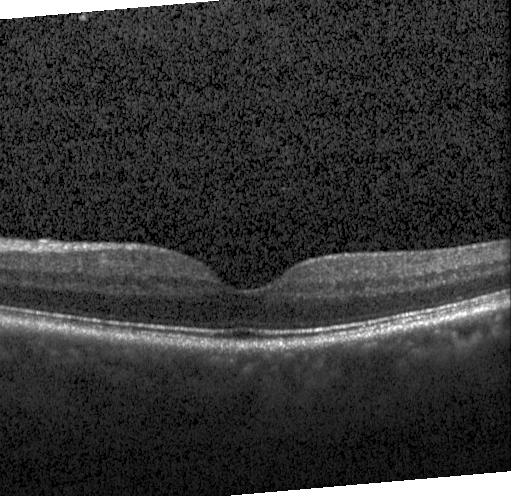

OCT line scan. Spectral-domain OCT. Macular scan
Finding: no evidence of choroidal neovascularization, diabetic macular edema, or drusen.